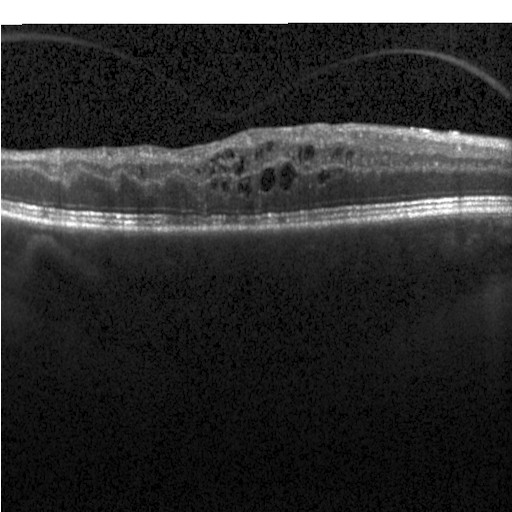 Optical coherence tomography B-scan; Heidelberg Spectralis; through the macula; spectral-domain optical coherence tomography — Diagnosis: diabetic macular edema.